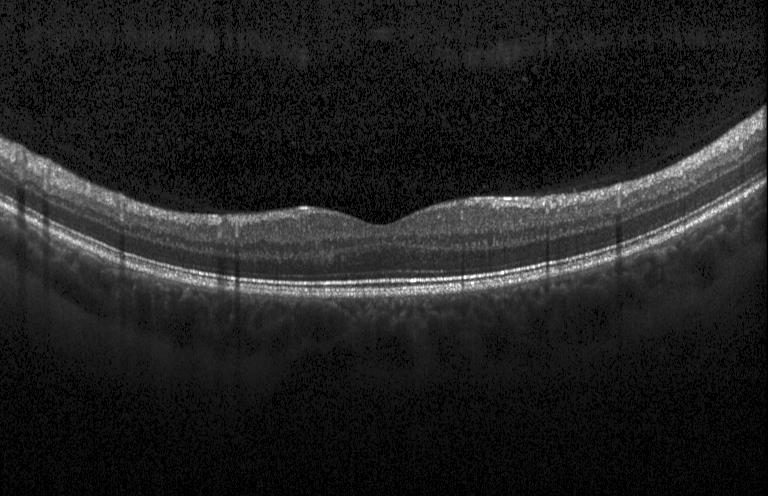
OCT line scan — Macular OCT: no evidence of choroidal neovascularization, diabetic macular edema, or drusen.